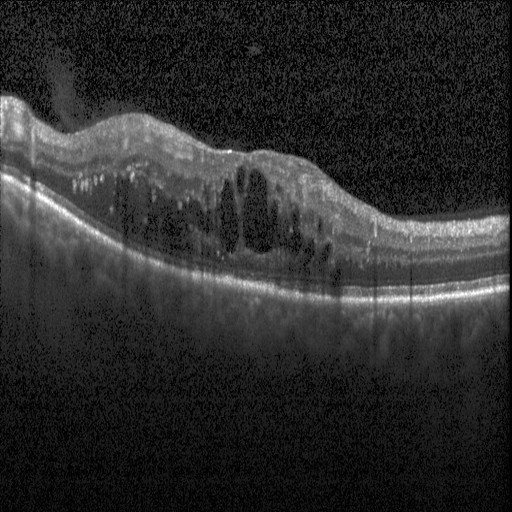
OCT B-scan
Diagnosis: DME.